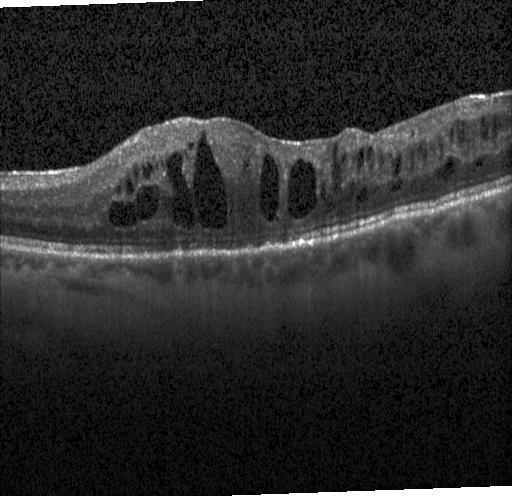

Dx: DME.